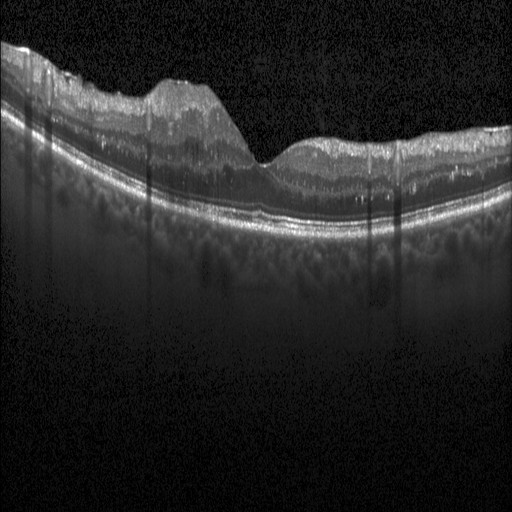
Macular OCT: DME.